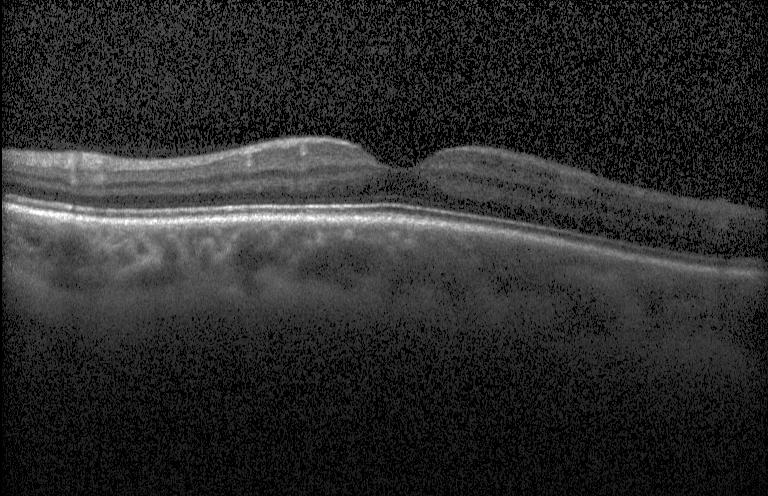 Retinal OCT B-scan
This B-scan demonstrates no CNV, no DME, and no drusen.